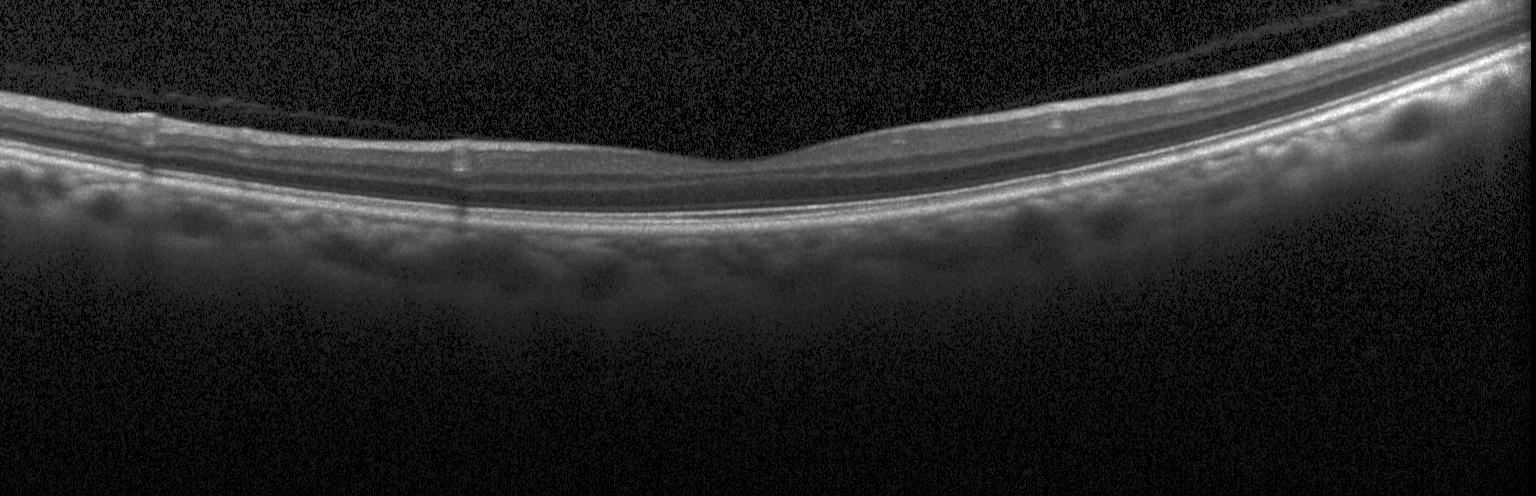
Macular OCT demonstrating no choroidal neovascularization, diabetic macular edema, or drusen.